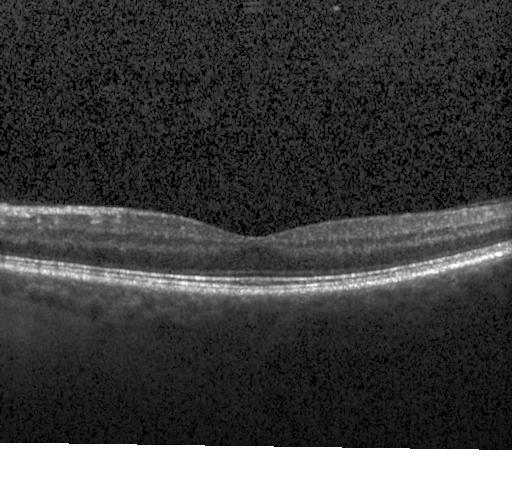 Diagnosis: neither choroidal neovascularization, diabetic macular edema, nor drusen.